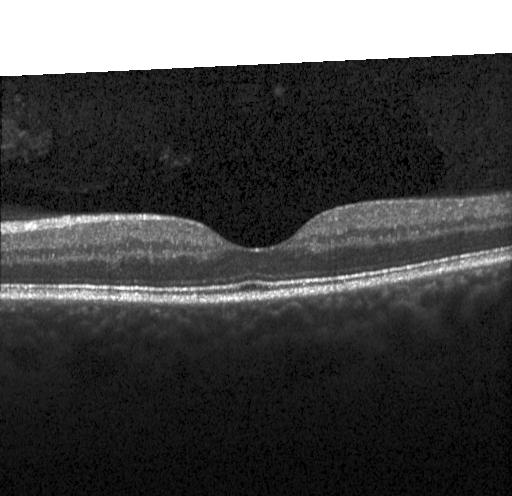

Spectral-domain OCT, optical coherence tomography scan, acquired on a Heidelberg Spectralis. The scan shows no choroidal neovascularization, no diabetic macular edema, and no drusen.